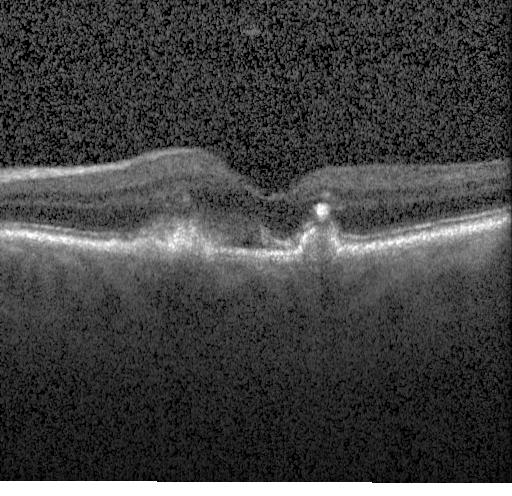
Retinal OCT cross-section · spectral-domain optical coherence tomography · Heidelberg Spectralis — Assessment: a choroidal neovascular membrane.